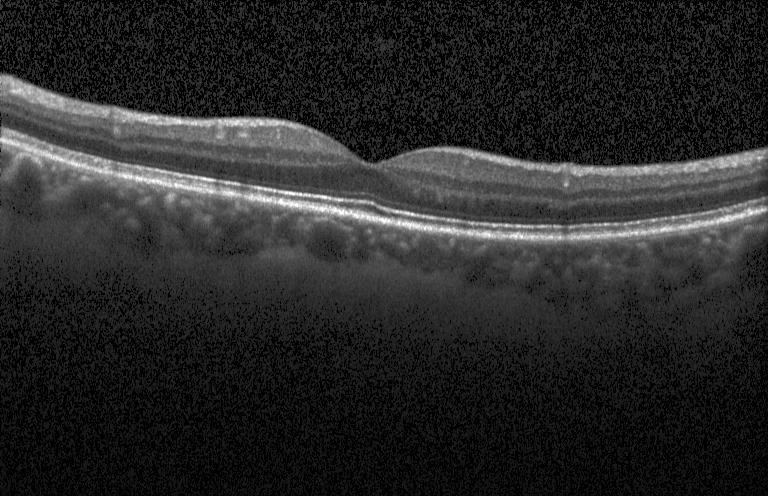

Optical coherence tomography B-scan — Macular OCT: no evidence of CNV, DME, or drusen.